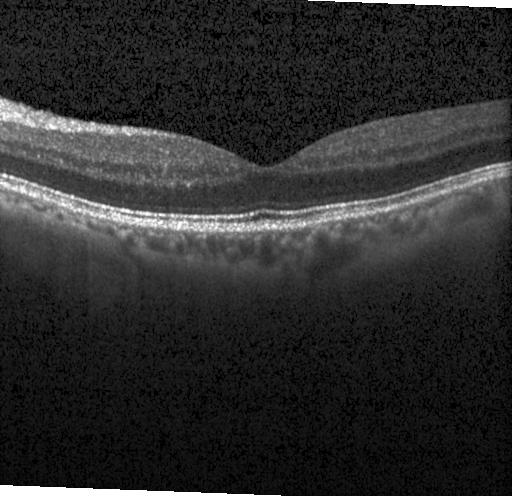 Retinal OCT cross-section
Impression: no choroidal neovascularization, diabetic macular edema, or drusen.